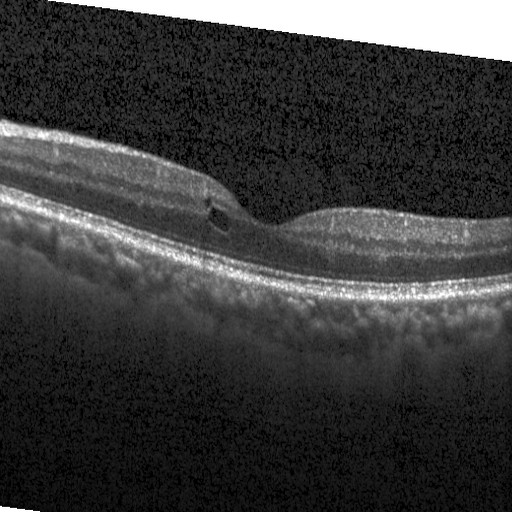

Macular OCT: diabetic macular edema (DME).